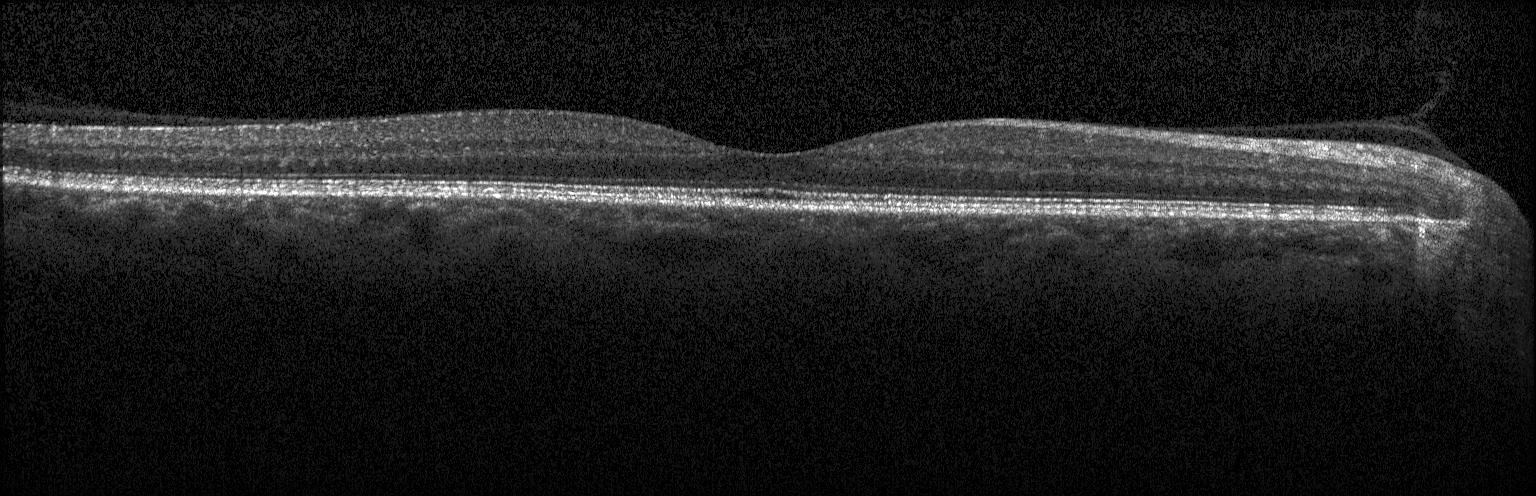 Macular OCT demonstrating neither choroidal neovascularization, diabetic macular edema, nor drusen.